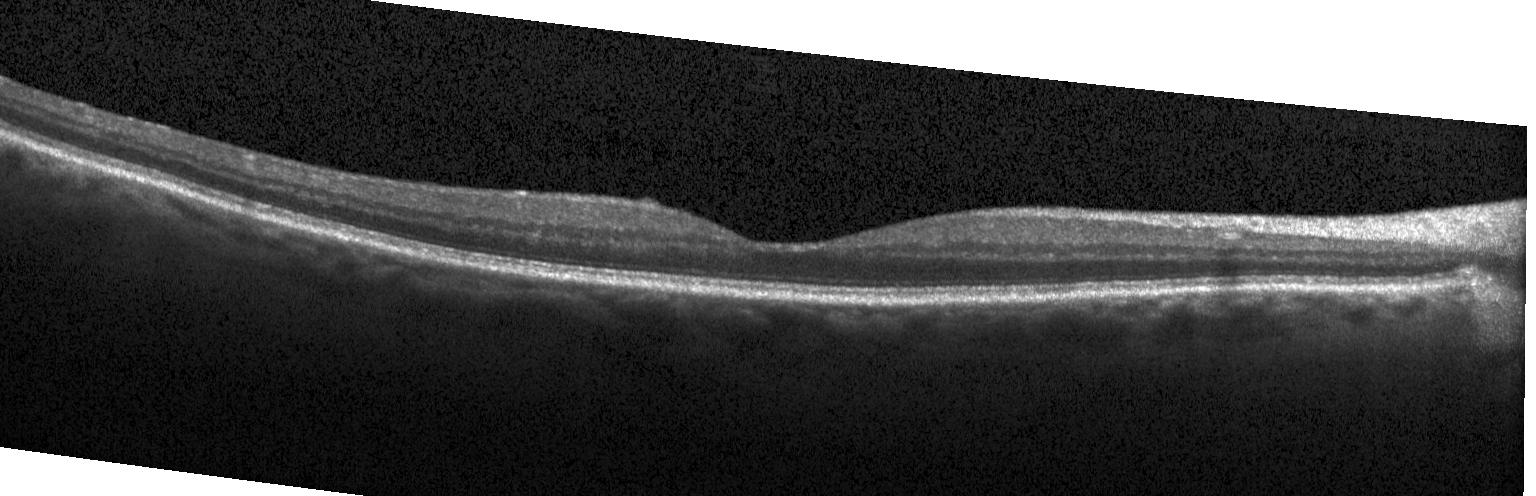 Centered on the fovea. Retinal OCT cross-section
Dx: no CNV, DME, or drusen.